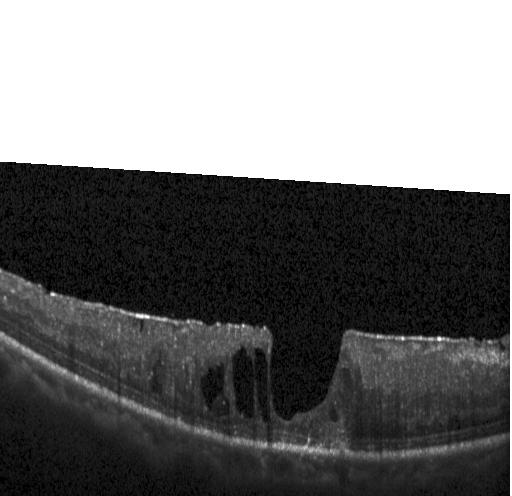
DME.